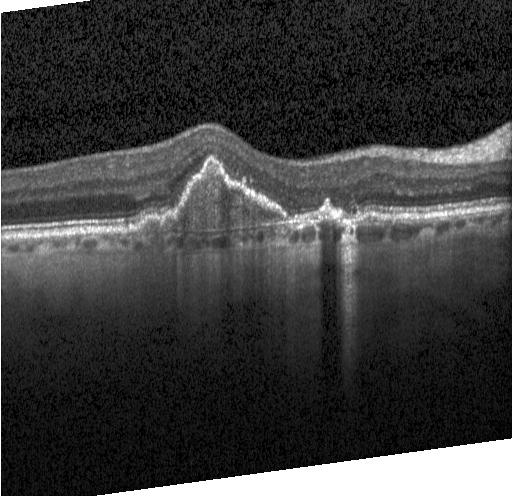 Spectral-domain optical coherence tomography · optical coherence tomography scan · macular scan. This B-scan demonstrates CNV.